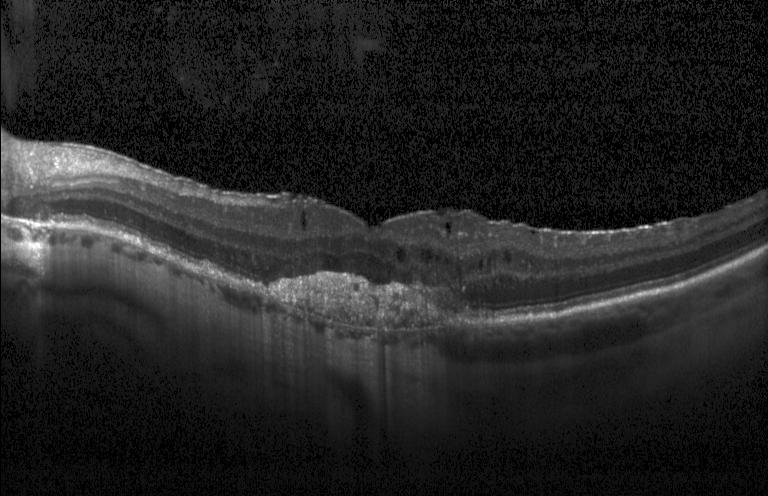
OCT B-scan. Spectral-domain OCT. Heidelberg Spectralis. Finding: a choroidal neovascular membrane.